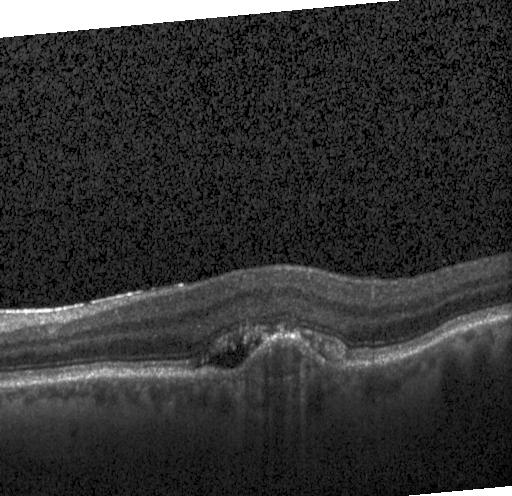
Fovea-centered. Spectral-domain OCT. Heidelberg Spectralis OCT system. Retinal OCT B-scan
A choroidal neovascular membrane.